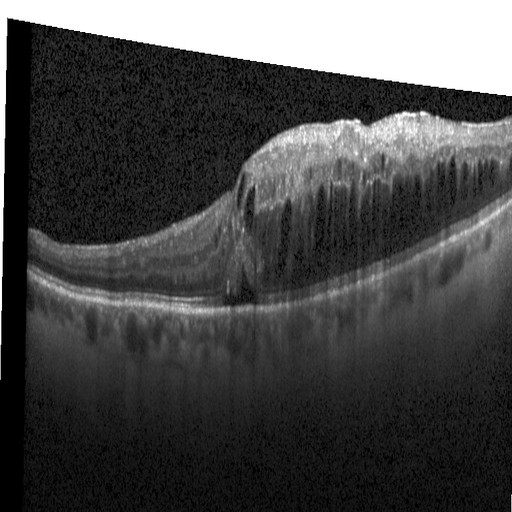

OCT finding: diabetic macular edema (DME).